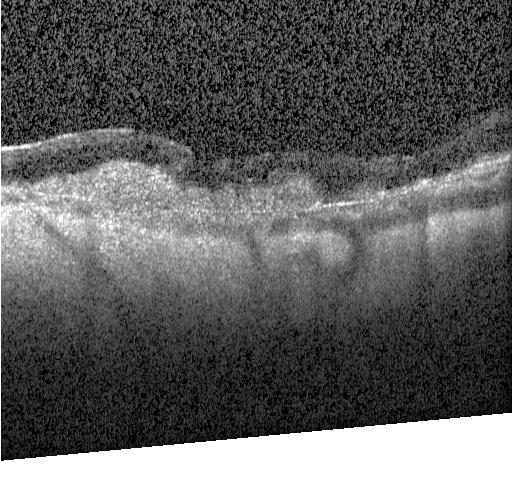 Instrument: Heidelberg Spectralis. Retinal OCT cross-section. Spectral-domain OCT.
Choroidal neovascularization (CNV).